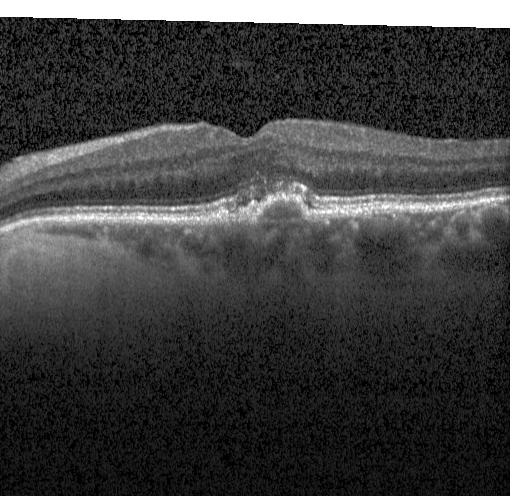

Optical coherence tomography scan — Finding: a choroidal neovascular membrane.